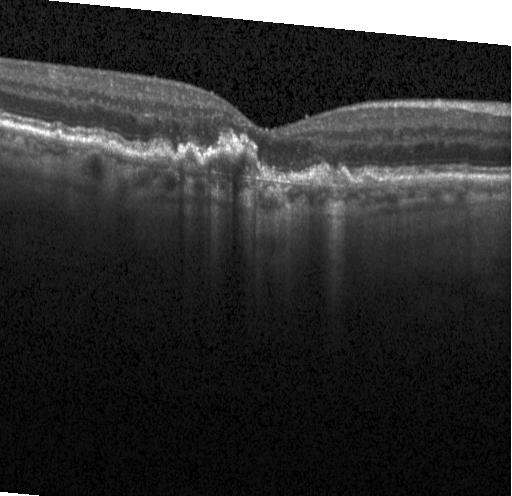 OCT line scan; SD-OCT; centered on the fovea. Assessment: CNV.